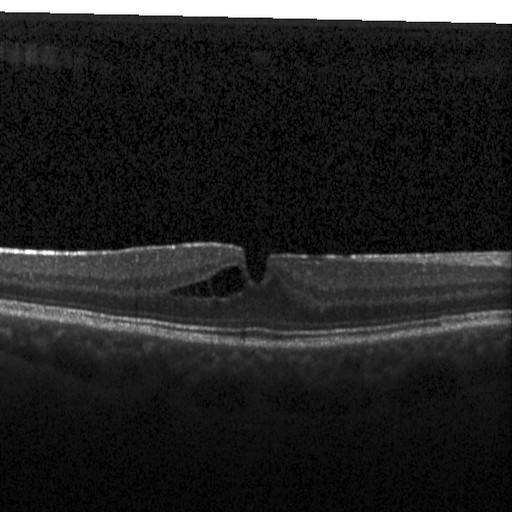
This B-scan demonstrates DME.